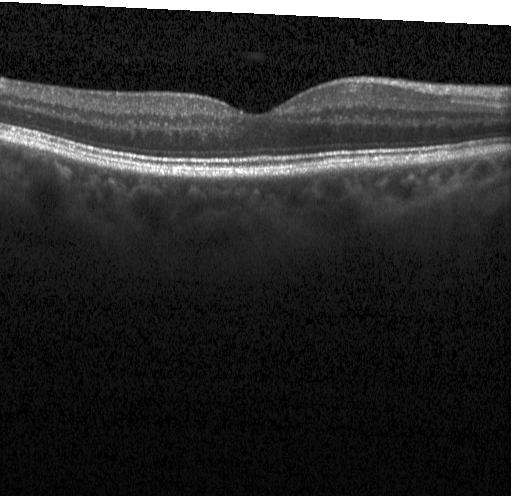

Acquired on a Heidelberg Spectralis · optical coherence tomography B-scan · spectral-domain optical coherence tomography · macular scan — Assessment: no choroidal neovascularization, diabetic macular edema, or drusen.